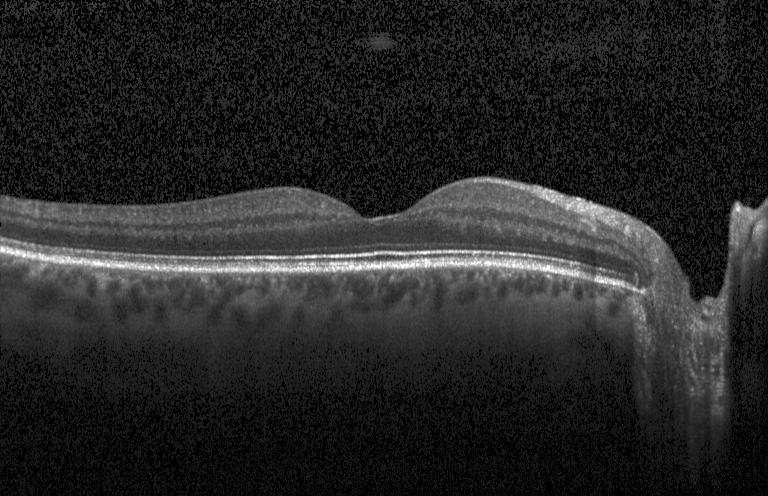
SD-OCT · OCT line scan · Heidelberg Spectralis OCT system · horizontal scan through the fovea — Impression: no choroidal neovascularization, no diabetic macular edema, and no drusen.